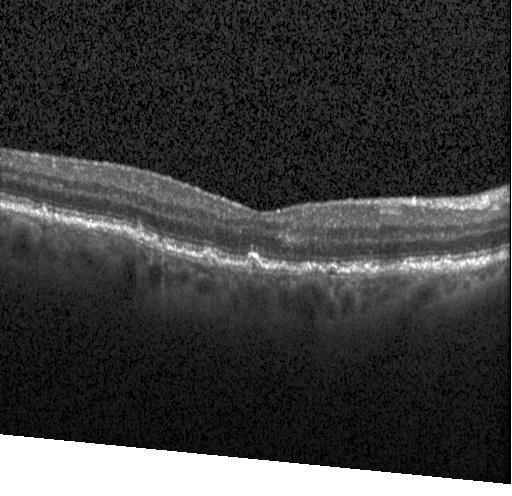
Finding: multiple drusen.